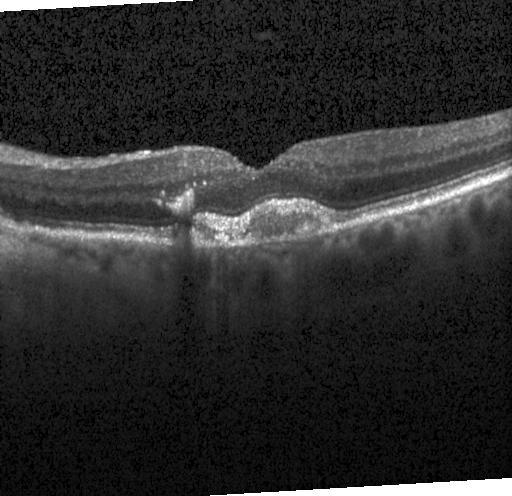

Horizontal scan through the fovea; acquired on a Heidelberg Spectralis; spectral-domain optical coherence tomography; optical coherence tomography scan.
The scan shows CNV.